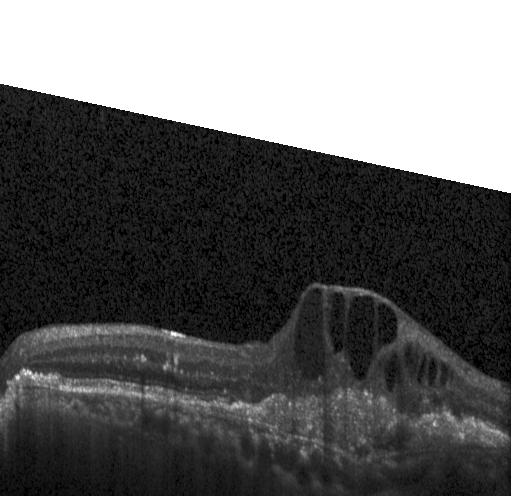 Retinal OCT cross-section showing a choroidal neovascular membrane.